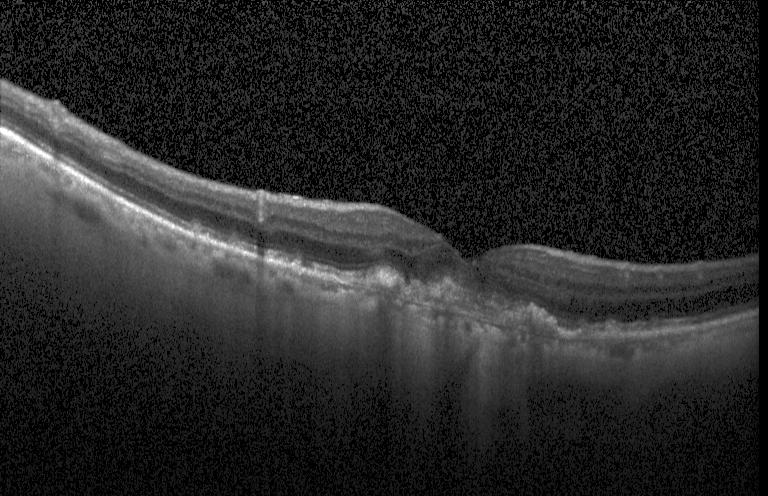 Acquired on a Heidelberg Spectralis; retinal OCT cross-section; centered on the fovea; spectral-domain OCT. Impression: a choroidal neovascular membrane.